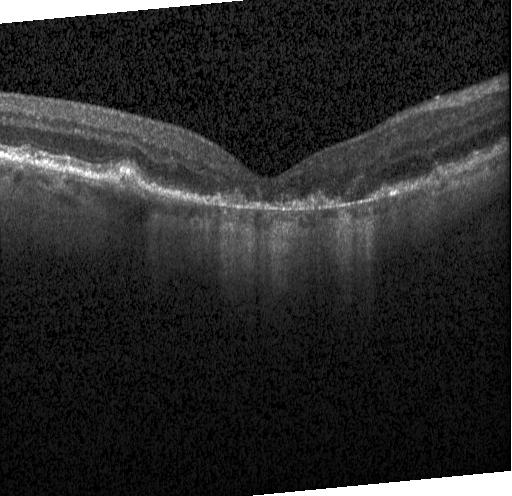
Macular OCT demonstrating CNV.